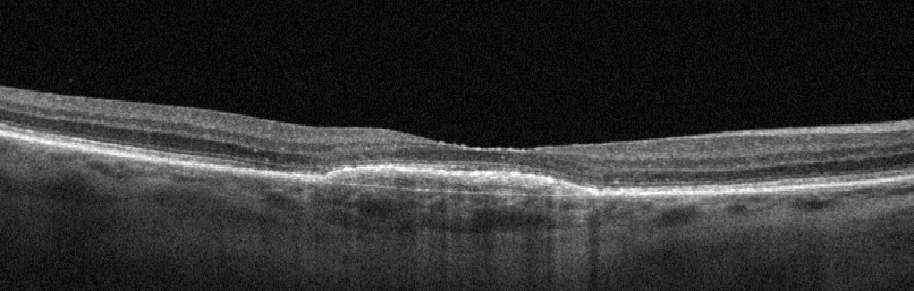

Through the macula, right eye, OCT B-scan.
Finding: age-related macular degeneration.